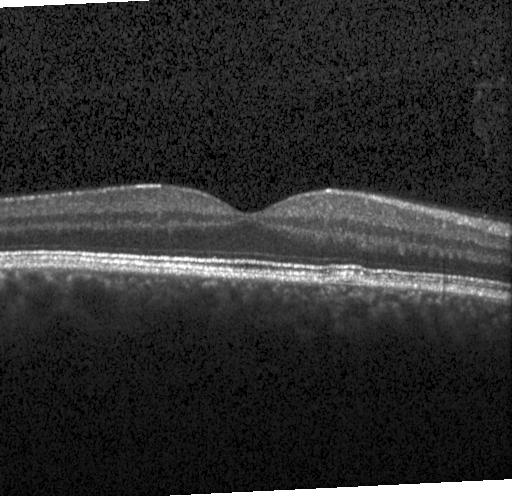

Heidelberg Spectralis. Optical coherence tomography scan. Macular scan. Spectral-domain OCT.
The scan shows neither choroidal neovascularization, diabetic macular edema, nor drusen.